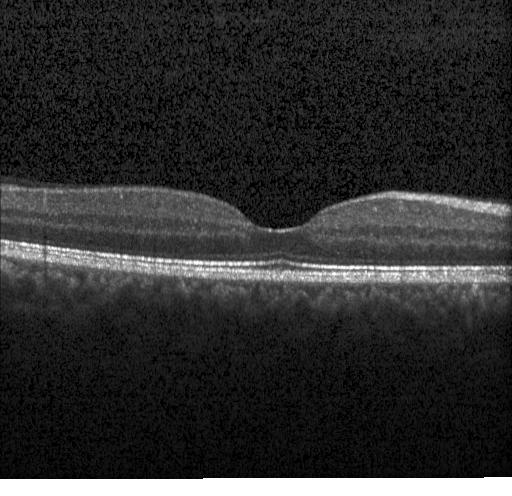 OCT finding: neither choroidal neovascularization, diabetic macular edema, nor drusen.